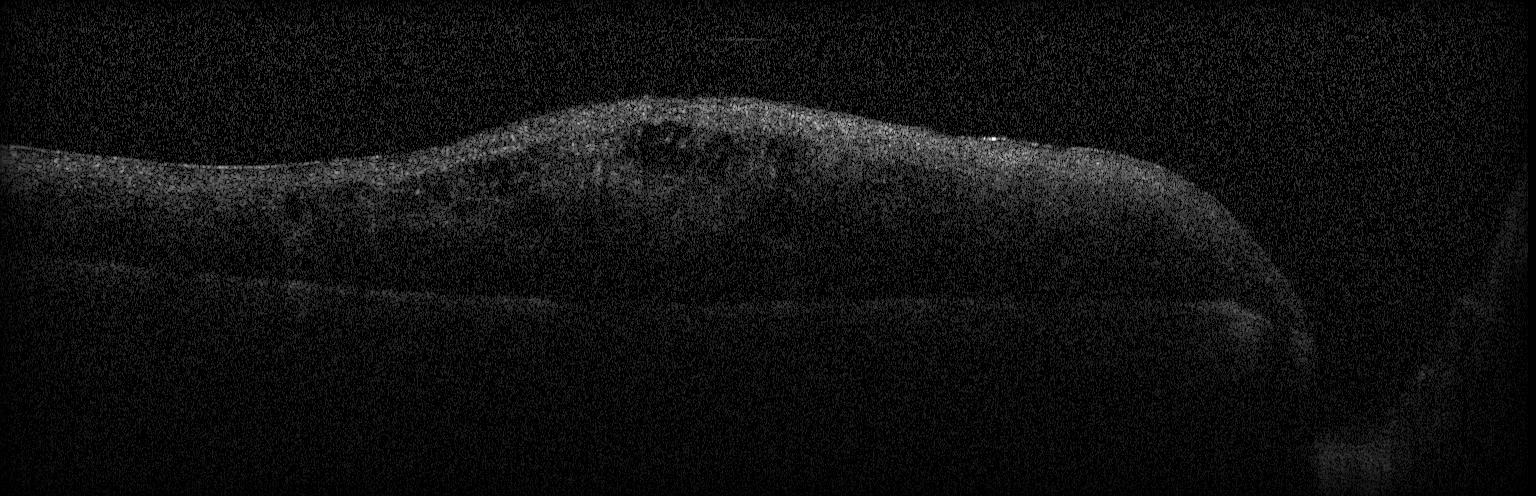 Heidelberg Spectralis OCT system. Retinal OCT B-scan — DME.